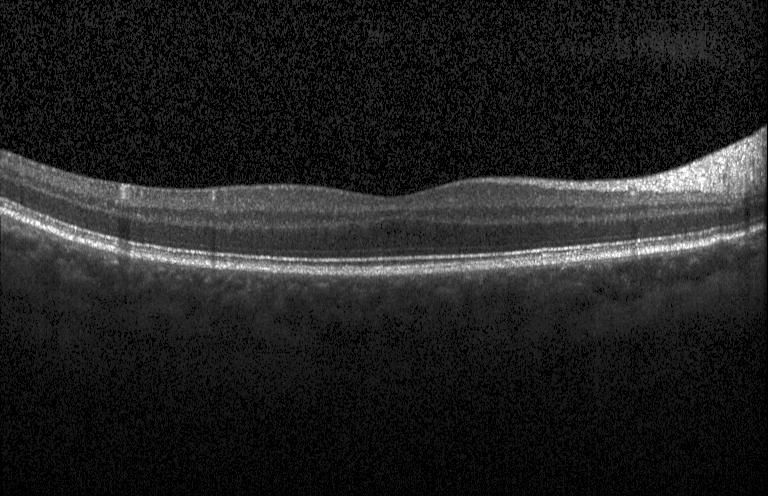 Impression: no CNV, no DME, and no drusen.